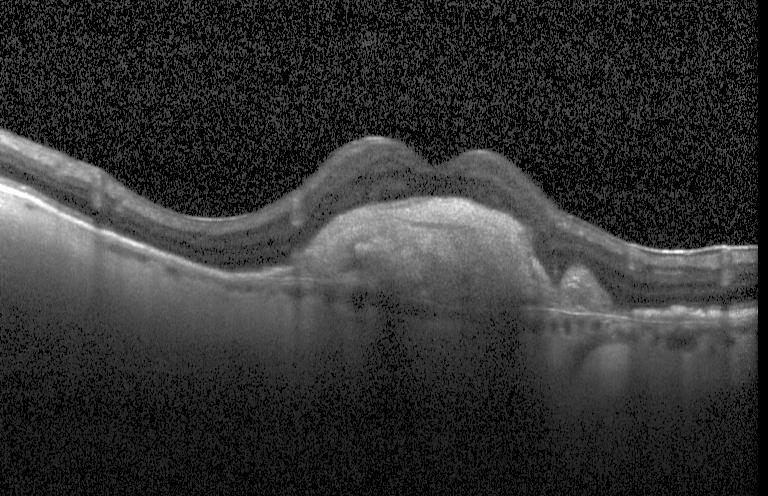

A choroidal neovascular membrane.